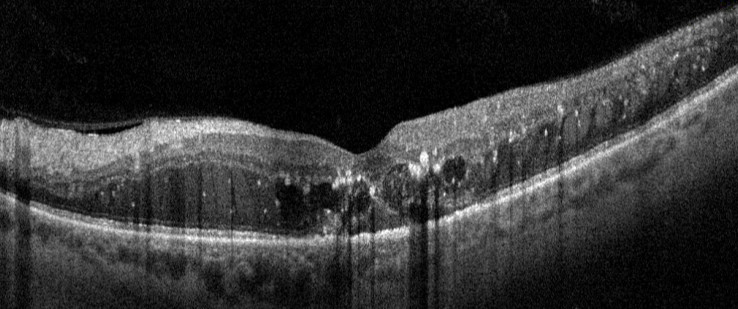
Through the macula. Retinal OCT B-scan. Acquired on an Optovue Avanti RTVue XR
Finding: diabetic macular edema.